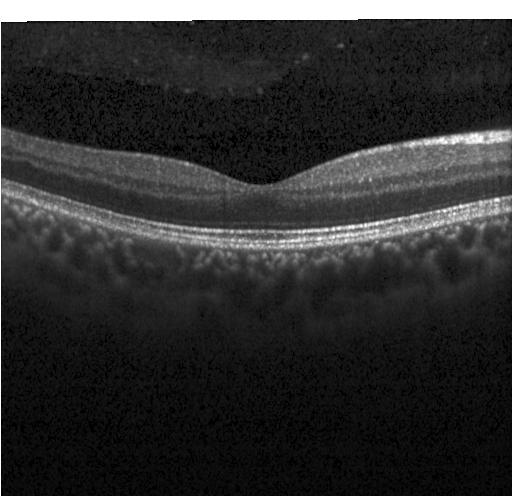

OCT B-scan — OCT finding: no choroidal neovascularization, no diabetic macular edema, and no drusen.